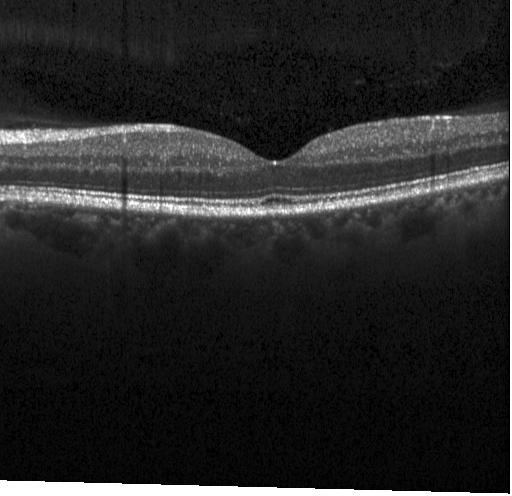

The scan shows neither choroidal neovascularization, diabetic macular edema, nor drusen.